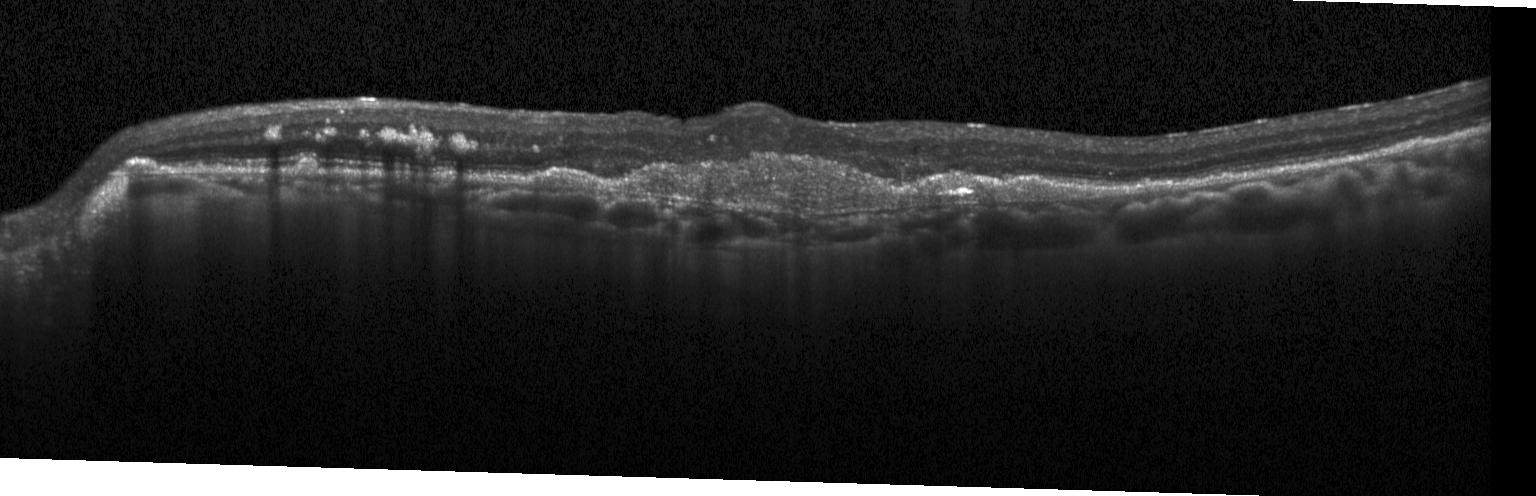

OCT B-scan showing choroidal neovascularization (CNV).